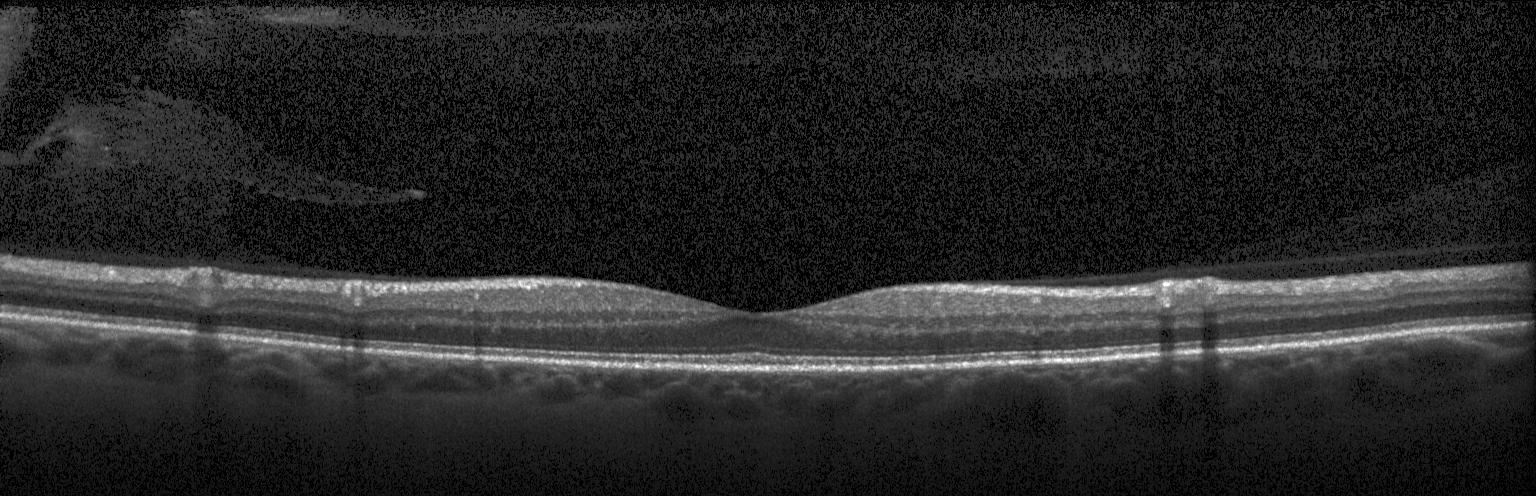

Finding: no evidence of choroidal neovascularization, diabetic macular edema, or drusen.